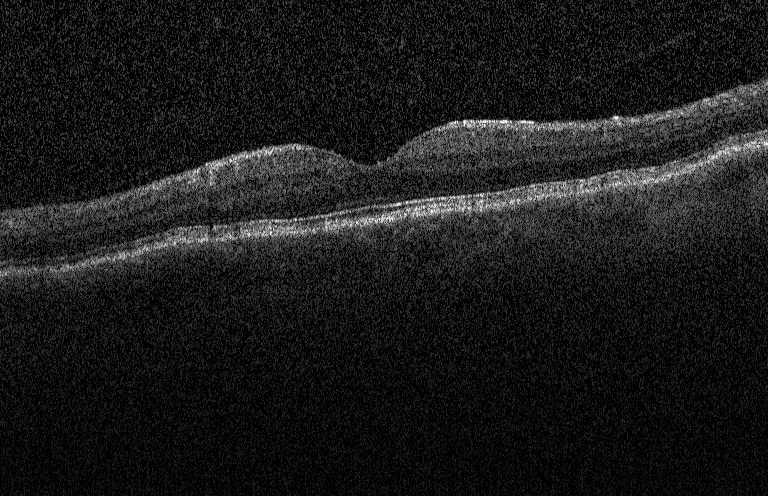 Spectral-domain optical coherence tomography, retinal OCT B-scan. Finding: neither choroidal neovascularization, diabetic macular edema, nor drusen.